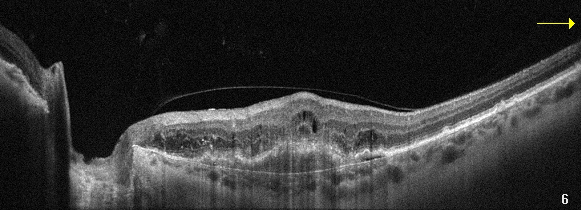 Finding: age-related macular degeneration (AMD).